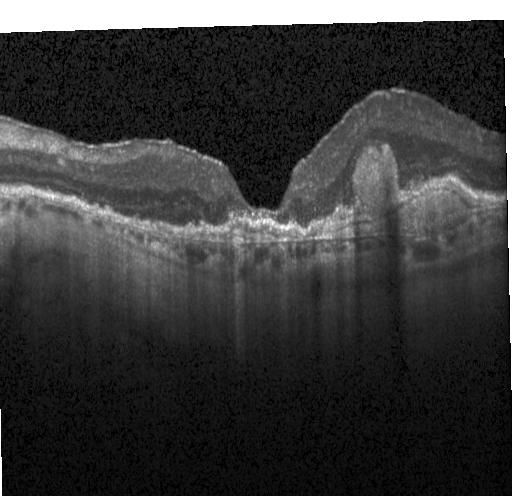
OCT B-scan showing a choroidal neovascular membrane.